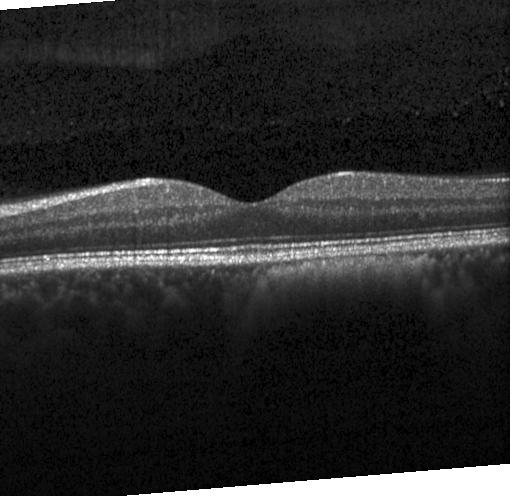 Dx: neither choroidal neovascularization, diabetic macular edema, nor drusen.